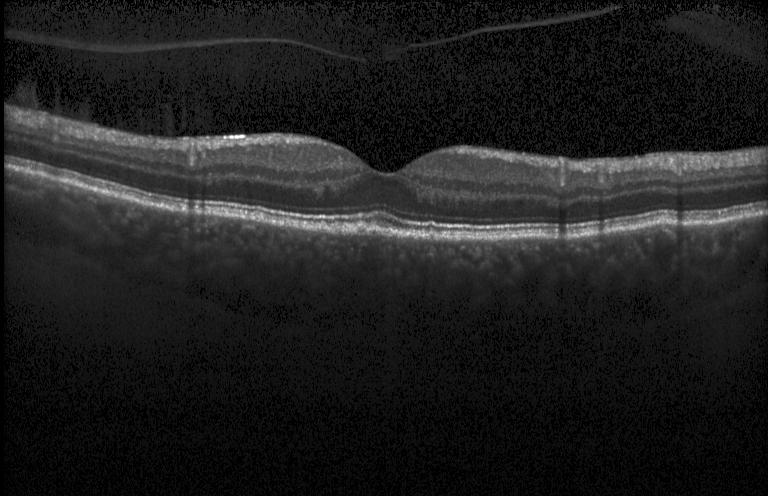

Optical coherence tomography B-scan; Heidelberg Spectralis OCT system.
Finding: drusen.